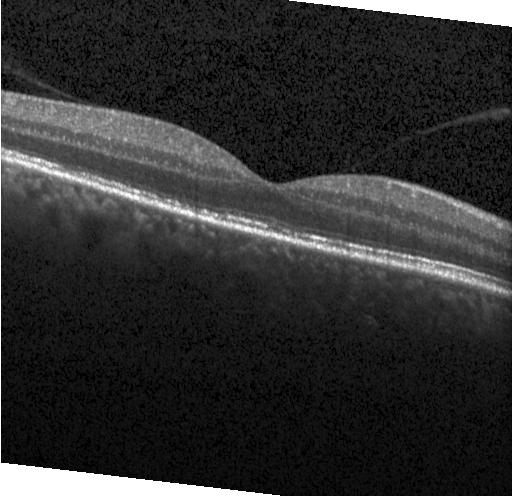

Impression: neither choroidal neovascularization, diabetic macular edema, nor drusen.